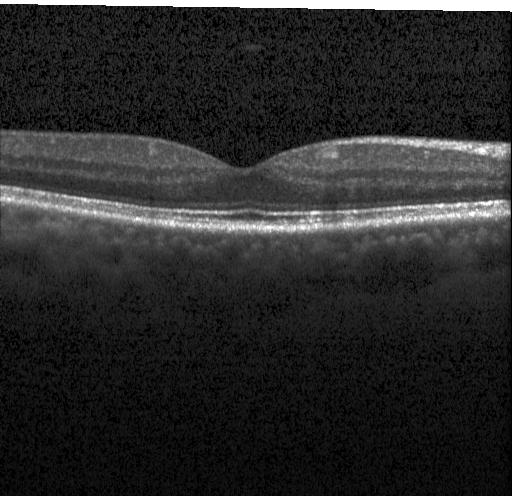
Retinal OCT cross-section showing no evidence of choroidal neovascularization, diabetic macular edema, or drusen.